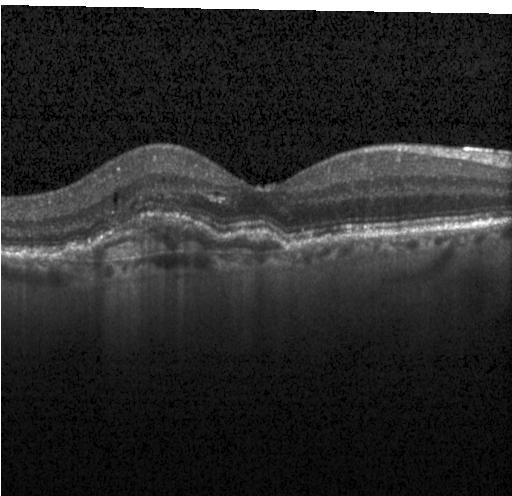

Dx: a choroidal neovascular membrane.